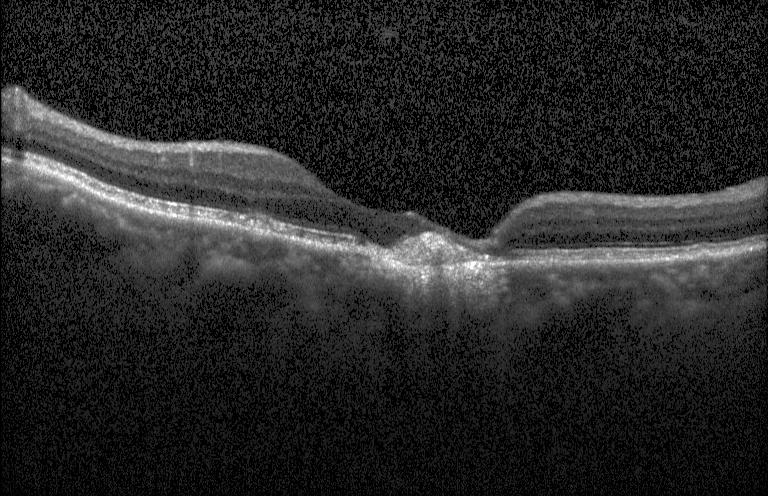 Retinal OCT B-scan.
Assessment: a choroidal neovascular membrane.